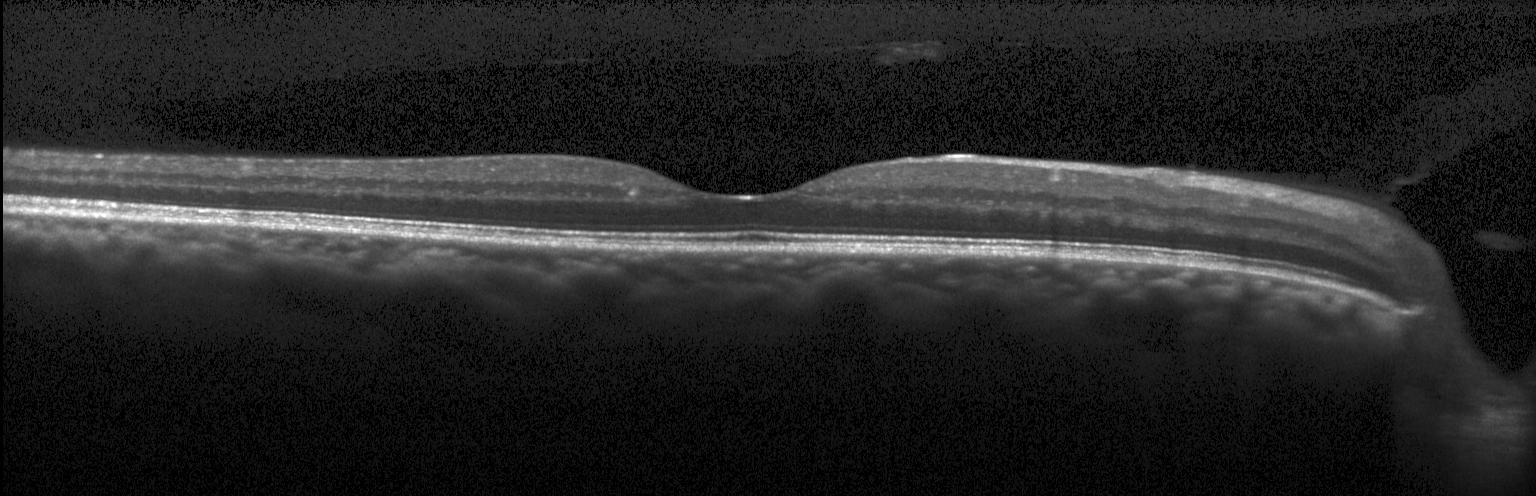

Retinal OCT B-scan · centered on the fovea · Heidelberg Spectralis OCT system · spectral-domain optical coherence tomography.
Assessment: no choroidal neovascularization, diabetic macular edema, or drusen.